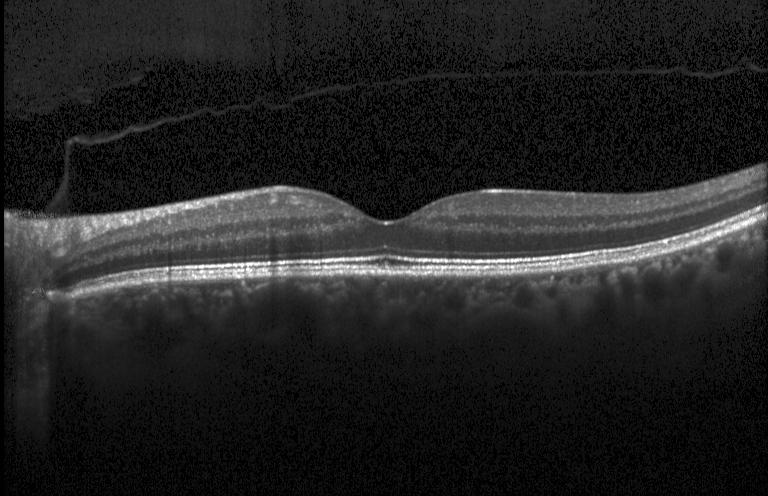 Heidelberg Spectralis; spectral-domain OCT; retinal OCT B-scan; centered on the fovea.
This B-scan demonstrates no choroidal neovascularization, diabetic macular edema, or drusen.